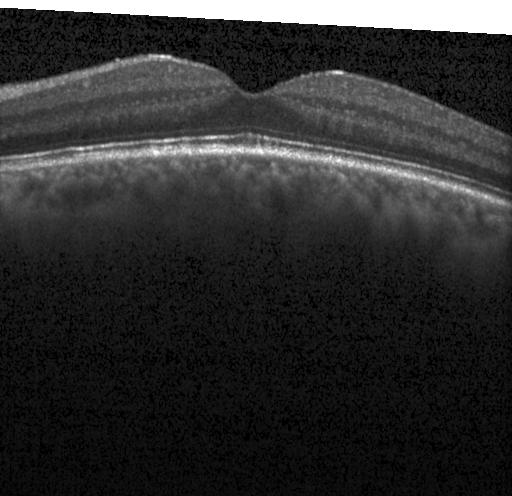

Diagnosis: no choroidal neovascularization, no diabetic macular edema, and no drusen.